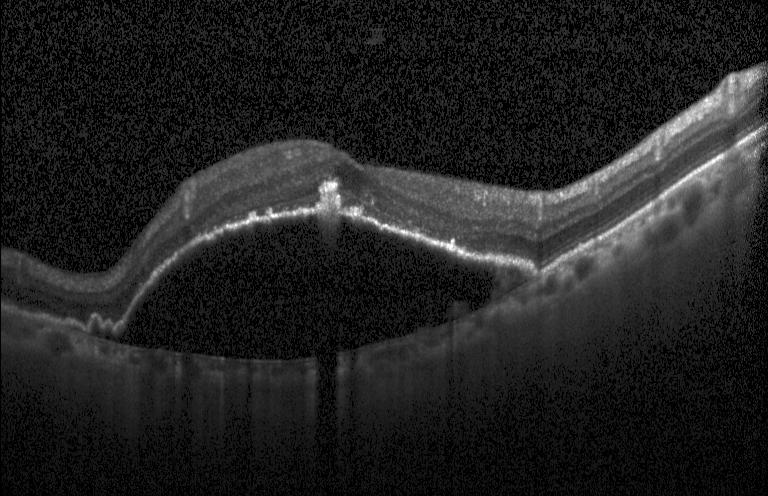
Heidelberg Spectralis, spectral-domain optical coherence tomography, horizontal scan through the fovea, OCT line scan
This B-scan demonstrates a choroidal neovascular membrane.